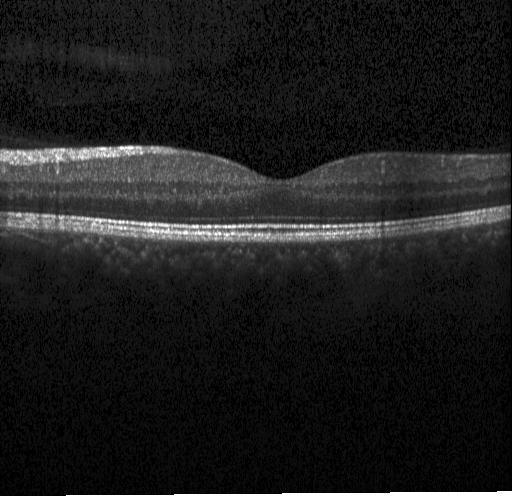
Optical coherence tomography B-scan
Macular OCT: no choroidal neovascularization, diabetic macular edema, or drusen.